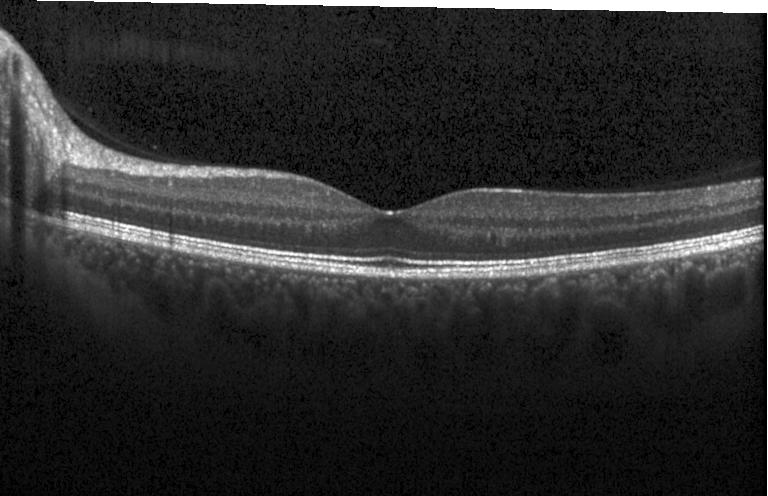 Spectral-domain OCT. Optical coherence tomography scan. Heidelberg Spectralis. Macular scan — Diagnosis: no choroidal neovascularization, no diabetic macular edema, and no drusen.